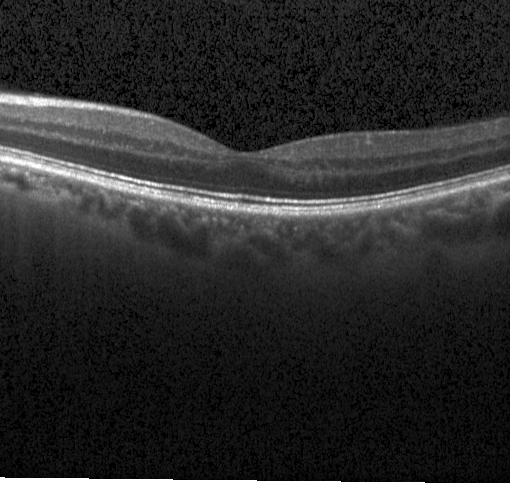

Heidelberg Spectralis OCT system. Optical coherence tomography B-scan. Macular scan. Spectral-domain OCT — Diagnosis: neither choroidal neovascularization, diabetic macular edema, nor drusen.